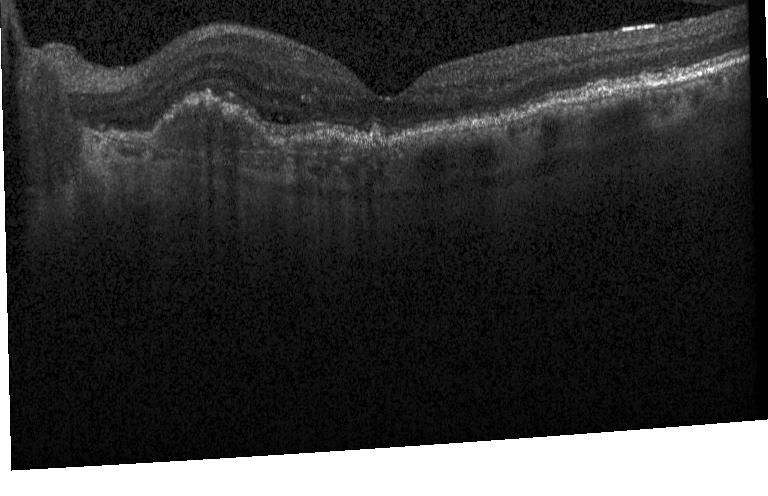

Macular OCT demonstrating choroidal neovascularization.